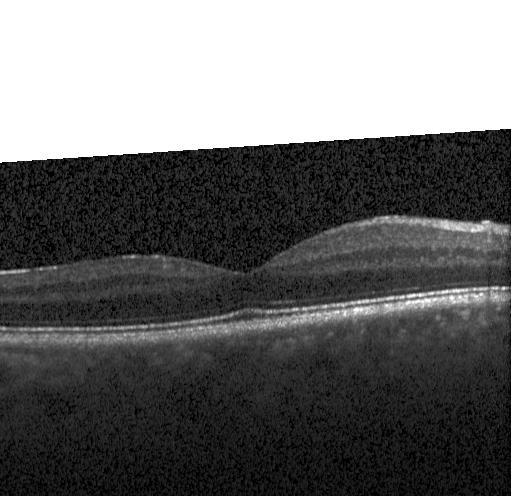 Finding: no CNV, DME, or drusen.